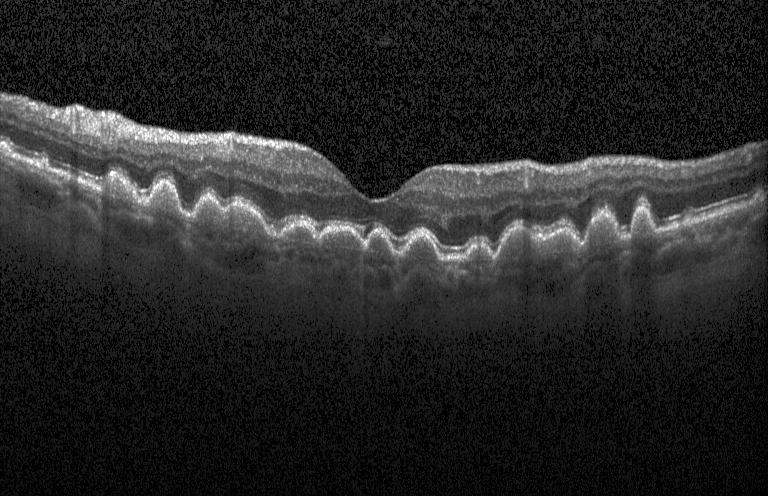
Finding: drusen.